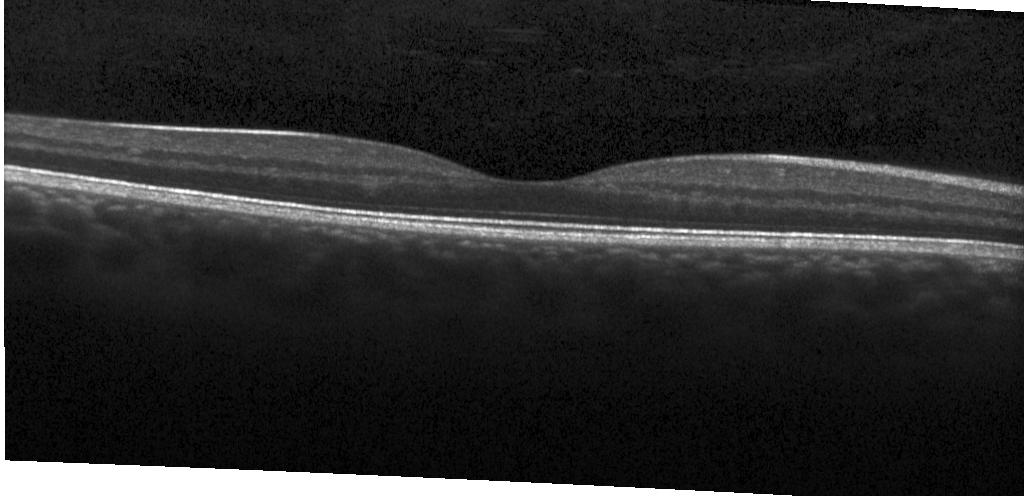

This B-scan demonstrates no choroidal neovascularization, diabetic macular edema, or drusen.